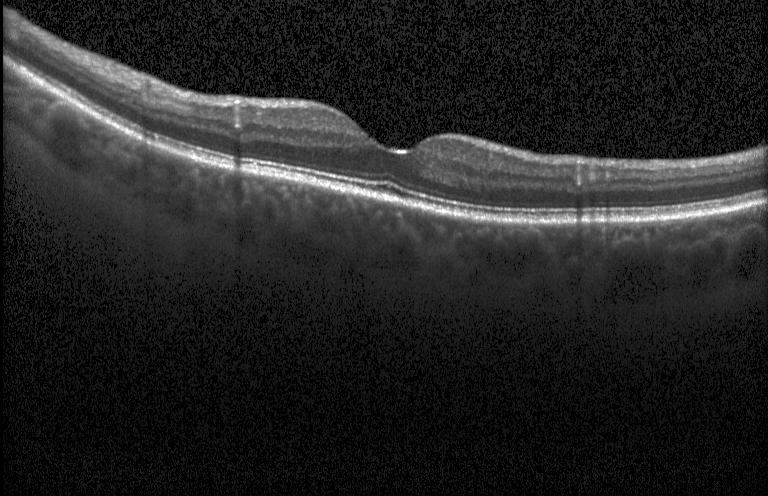 Spectral-domain optical coherence tomography · through the macula · instrument: Heidelberg Spectralis · retinal OCT cross-section. The scan shows no evidence of choroidal neovascularization, diabetic macular edema, or drusen.